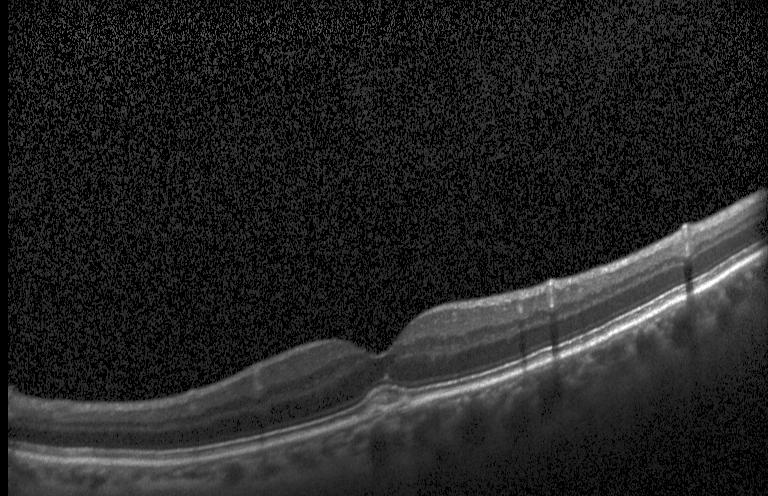 Through the macula; optical coherence tomography scan
Impression: CNV.